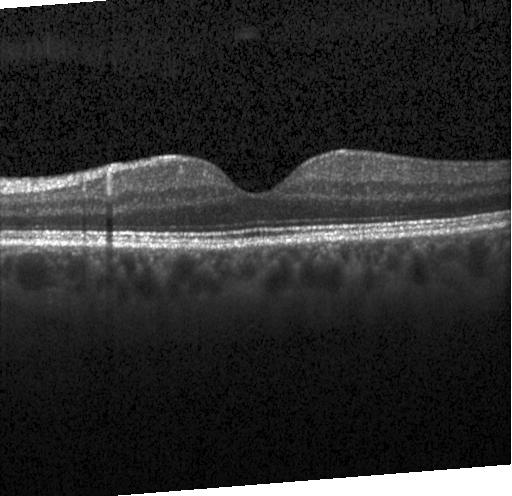
Retinal OCT B-scan · Heidelberg Spectralis
Assessment: no CNV, DME, or drusen.